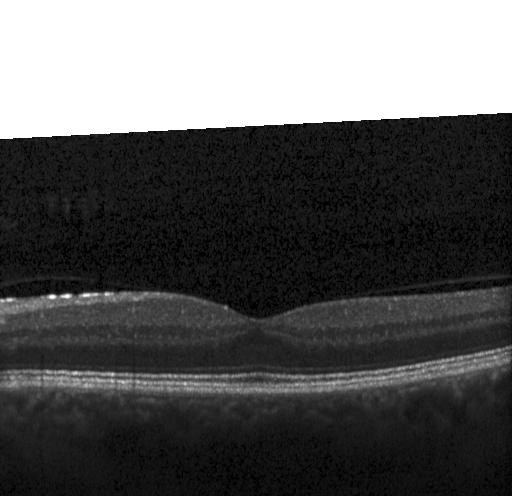 Heidelberg Spectralis OCT system. Retinal OCT cross-section
Impression: no choroidal neovascularization, diabetic macular edema, or drusen.